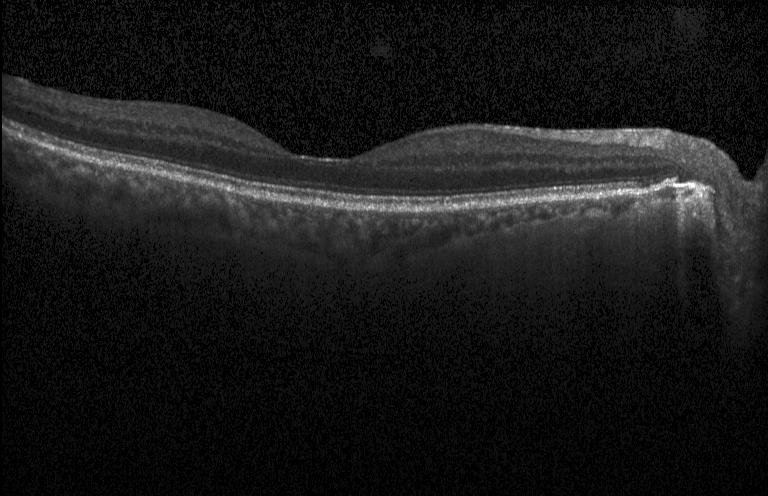 Finding: no choroidal neovascularization, no diabetic macular edema, and no drusen.